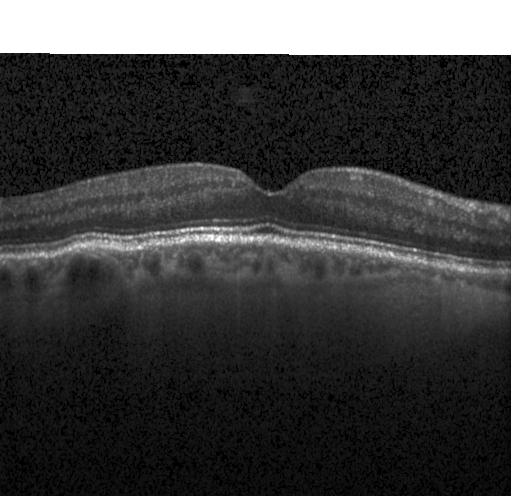

The scan shows neither CNV, DME, nor drusen.